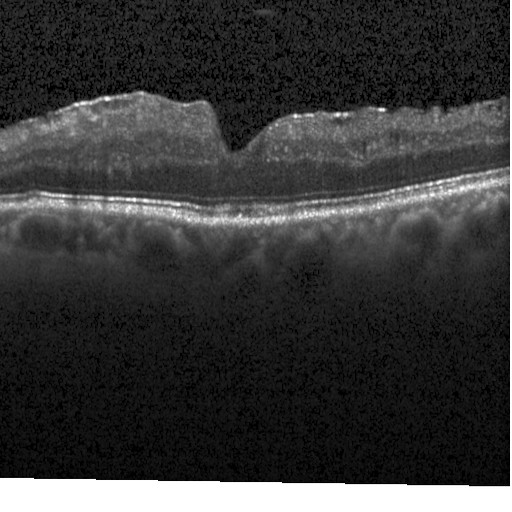

Finding: DME.